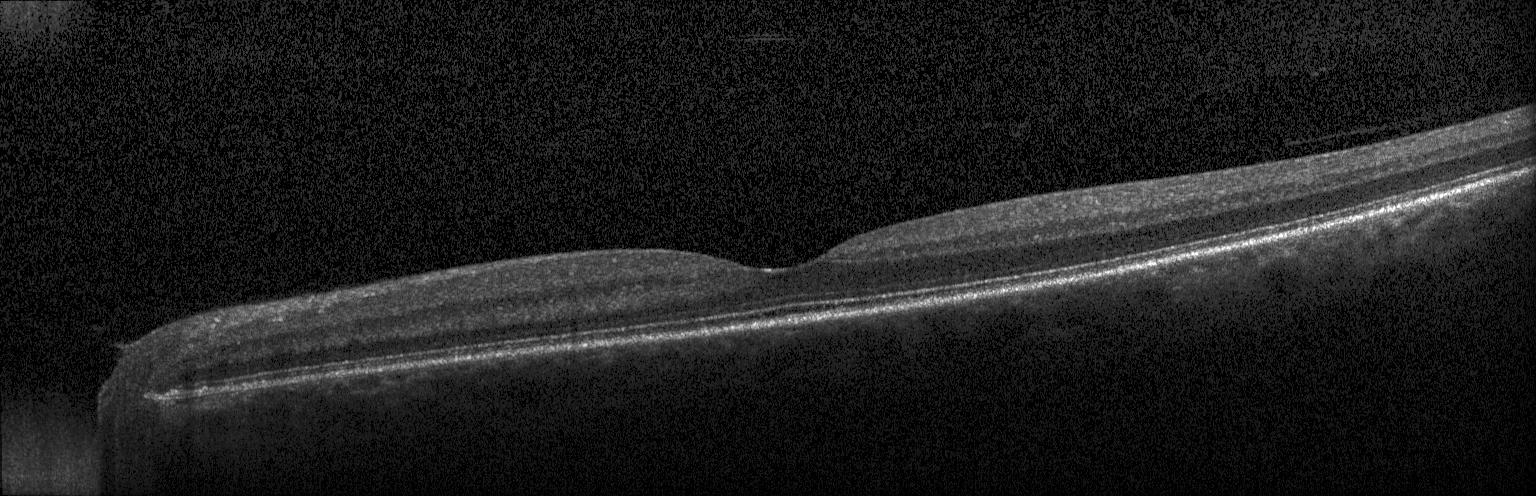

Impression: no choroidal neovascularization, diabetic macular edema, or drusen.